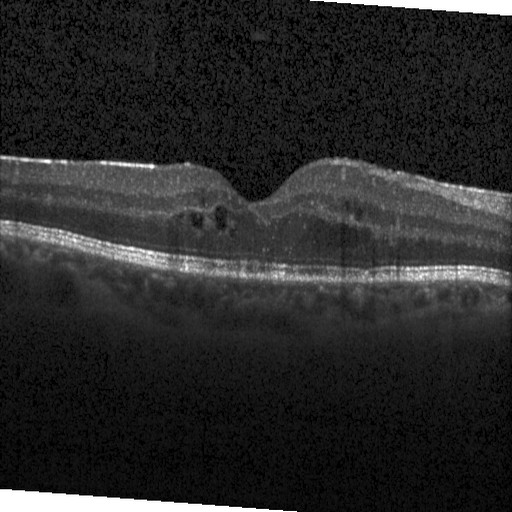 Instrument: Heidelberg Spectralis · OCT line scan.
Impression: DME.